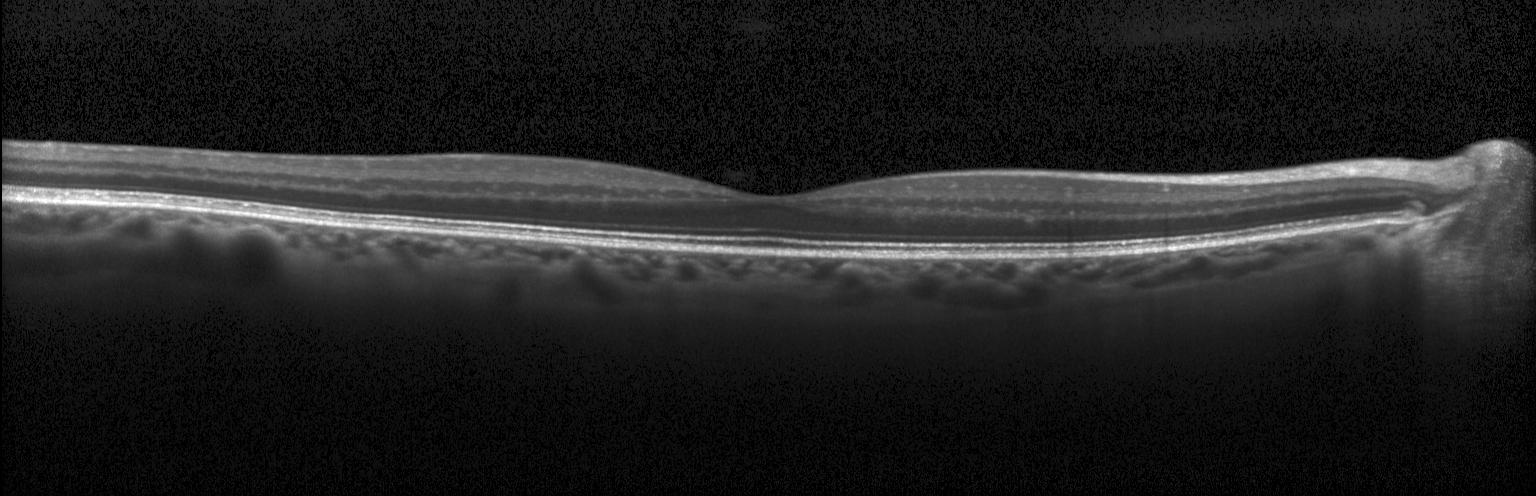

OCT scan showing neither choroidal neovascularization, diabetic macular edema, nor drusen.